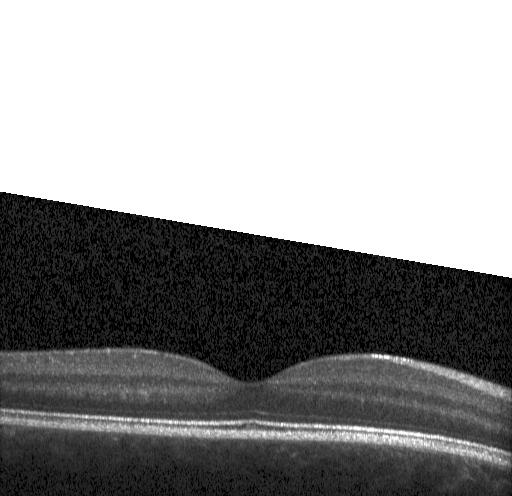
Impression: no CNV, no DME, and no drusen.